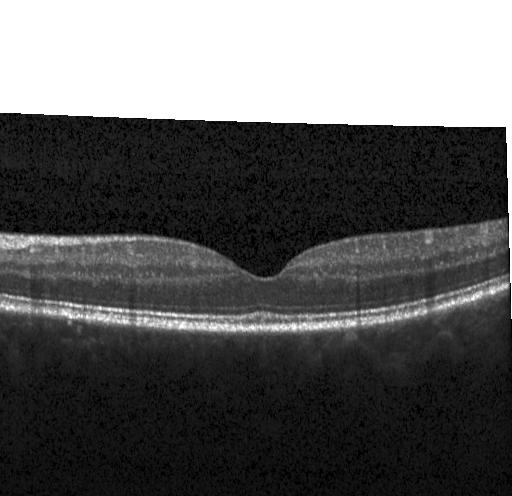 Heidelberg Spectralis OCT system. Spectral-domain OCT. Retinal OCT cross-section — Diagnosis: no choroidal neovascularization, no diabetic macular edema, and no drusen.